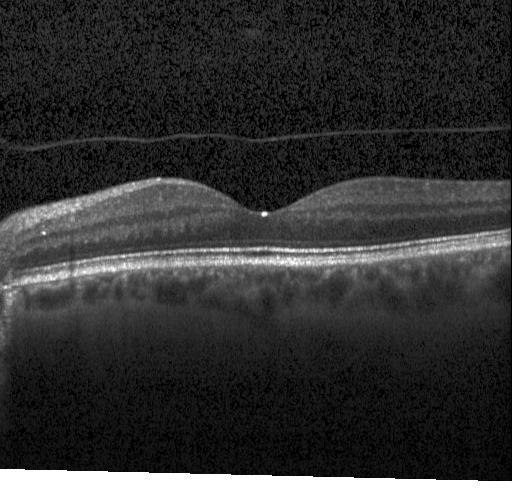

OCT line scan.
Finding: neither CNV, DME, nor drusen.